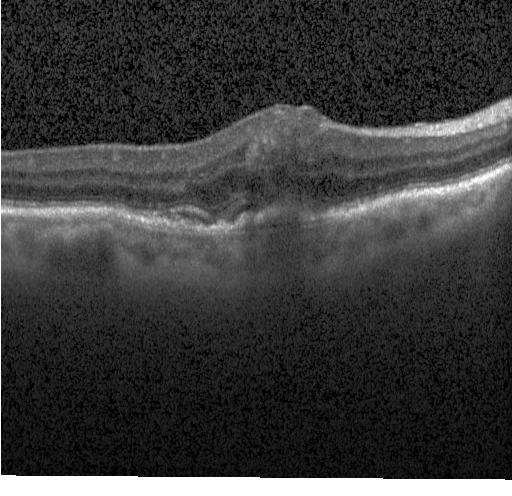
Impression: choroidal neovascularization (CNV).